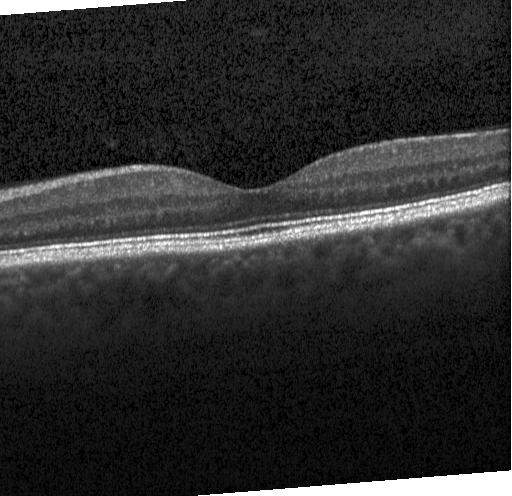 Heidelberg Spectralis; optical coherence tomography scan. Finding: no CNV, DME, or drusen.